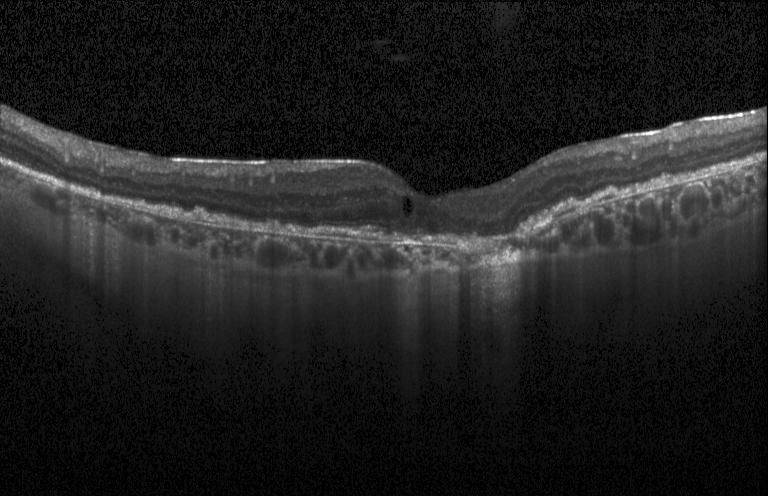 Dx: a choroidal neovascular membrane.